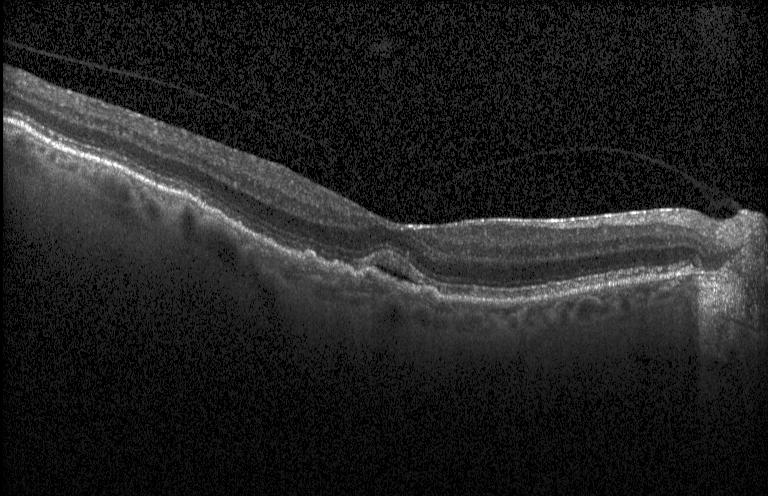 Impression: choroidal neovascularization (CNV).